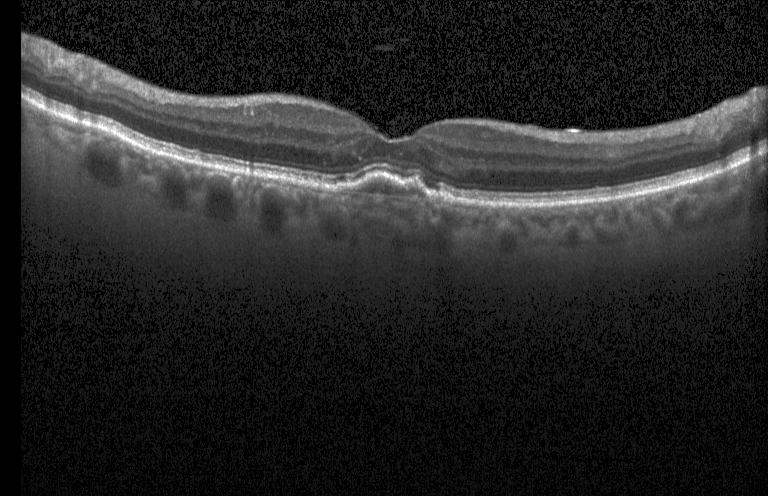

OCT finding: a choroidal neovascular membrane.